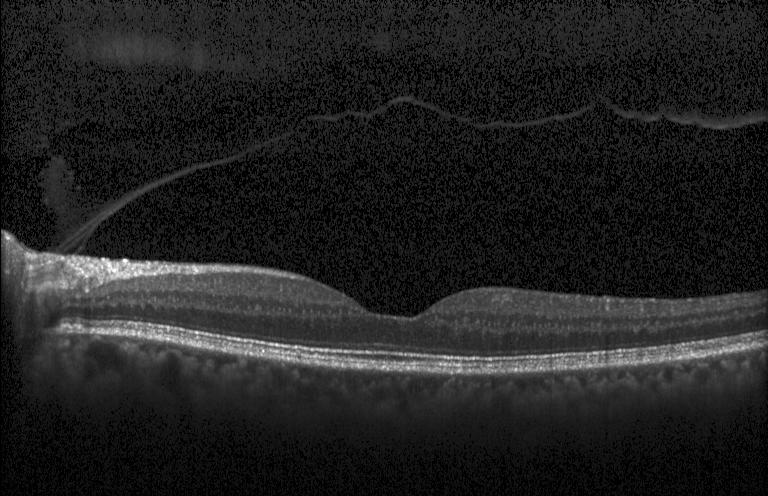 This B-scan demonstrates no evidence of choroidal neovascularization, diabetic macular edema, or drusen.